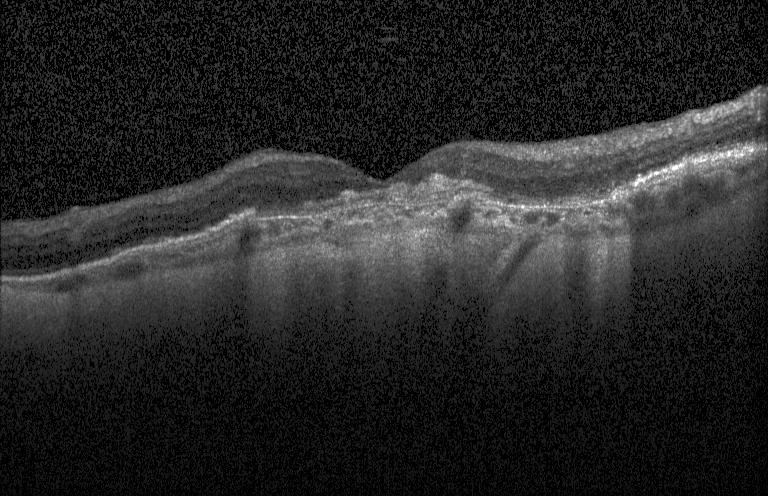

The scan shows a choroidal neovascular membrane.